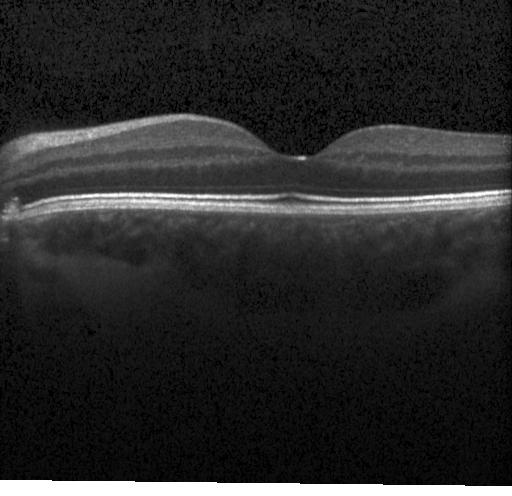

Macular OCT: no evidence of CNV, DME, or drusen.